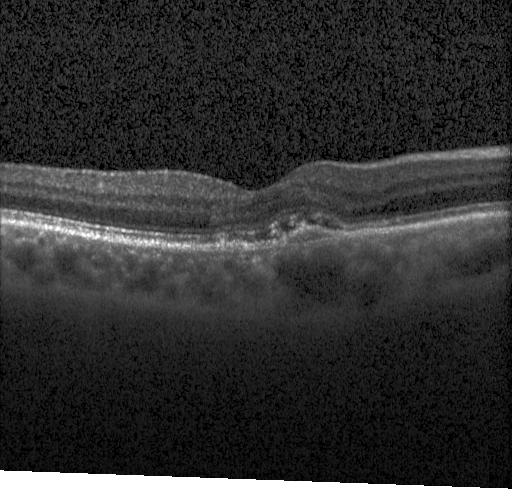

OCT B-scan
Finding: a choroidal neovascular membrane.